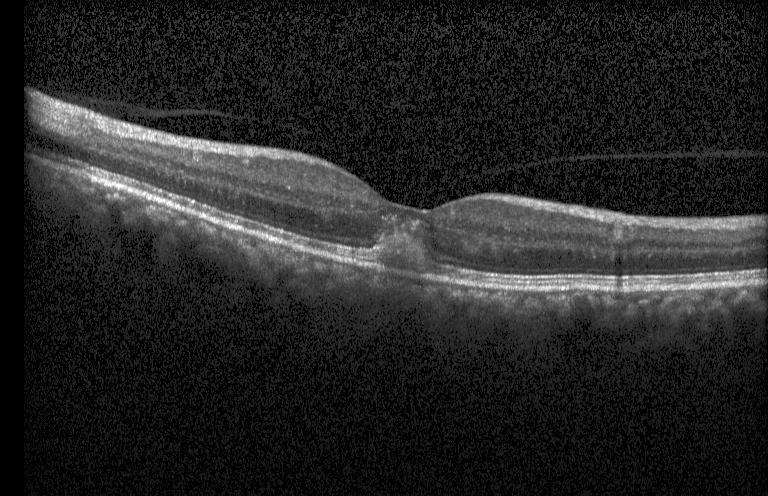
Retinal OCT B-scan, spectral-domain OCT, Heidelberg Spectralis OCT system, fovea-centered — Finding: choroidal neovascularization (CNV).